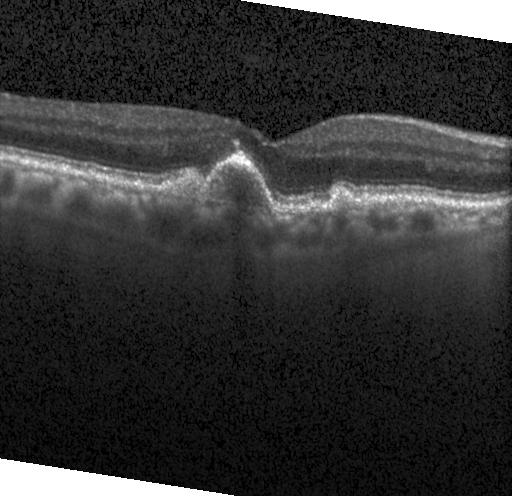

Optical coherence tomography B-scan.
Impression: sub-RPE drusenoid deposits.